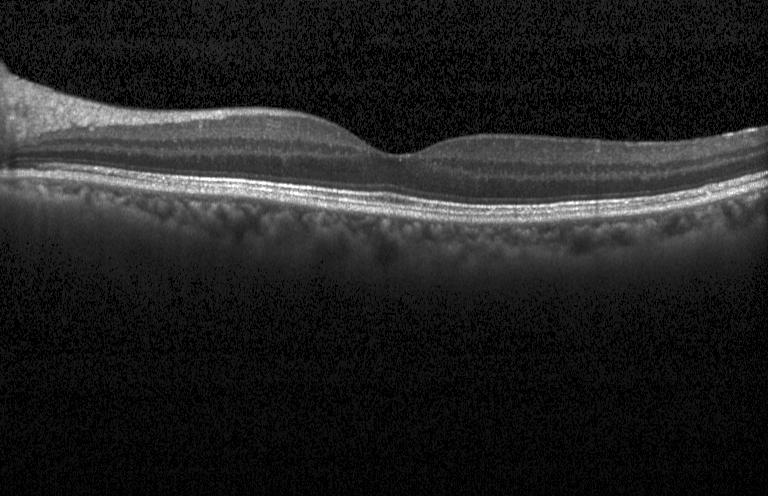

Retinal OCT B-scan — Impression: neither choroidal neovascularization, diabetic macular edema, nor drusen.